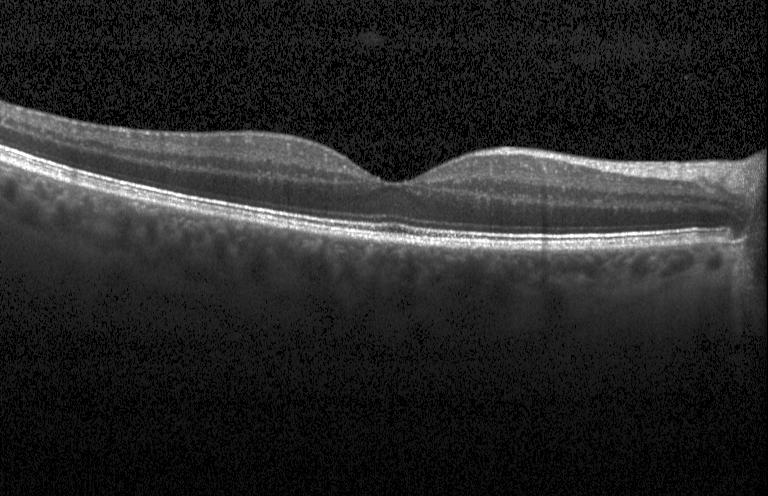

Heidelberg Spectralis, optical coherence tomography B-scan, fovea-centered, spectral-domain optical coherence tomography
Finding: no choroidal neovascularization, no diabetic macular edema, and no drusen.